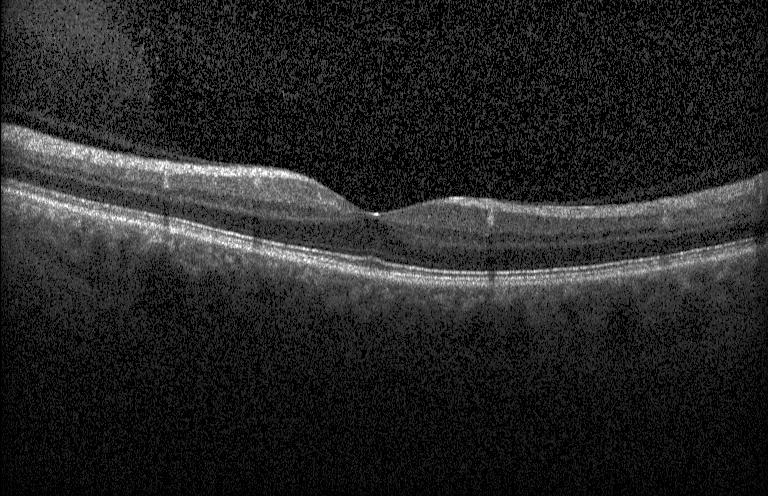

OCT finding: no evidence of CNV, DME, or drusen.